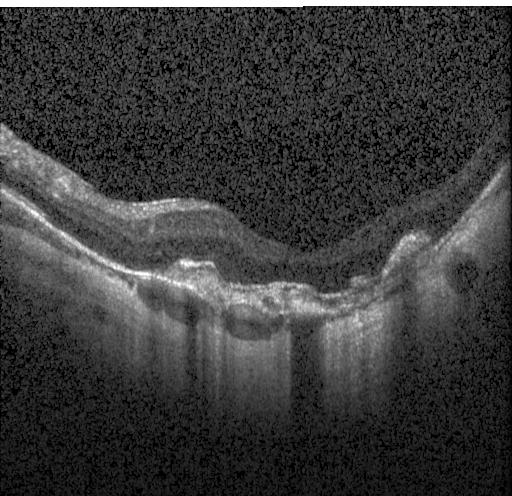
Heidelberg Spectralis, optical coherence tomography scan, through the macula, spectral-domain optical coherence tomography. This B-scan demonstrates a choroidal neovascular membrane.